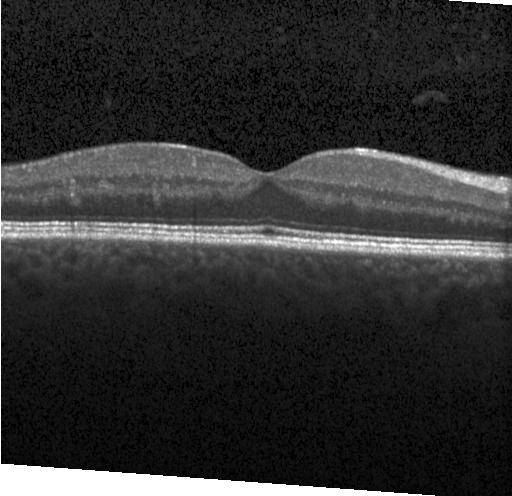 Optical coherence tomography scan. Impression: no choroidal neovascularization, diabetic macular edema, or drusen.